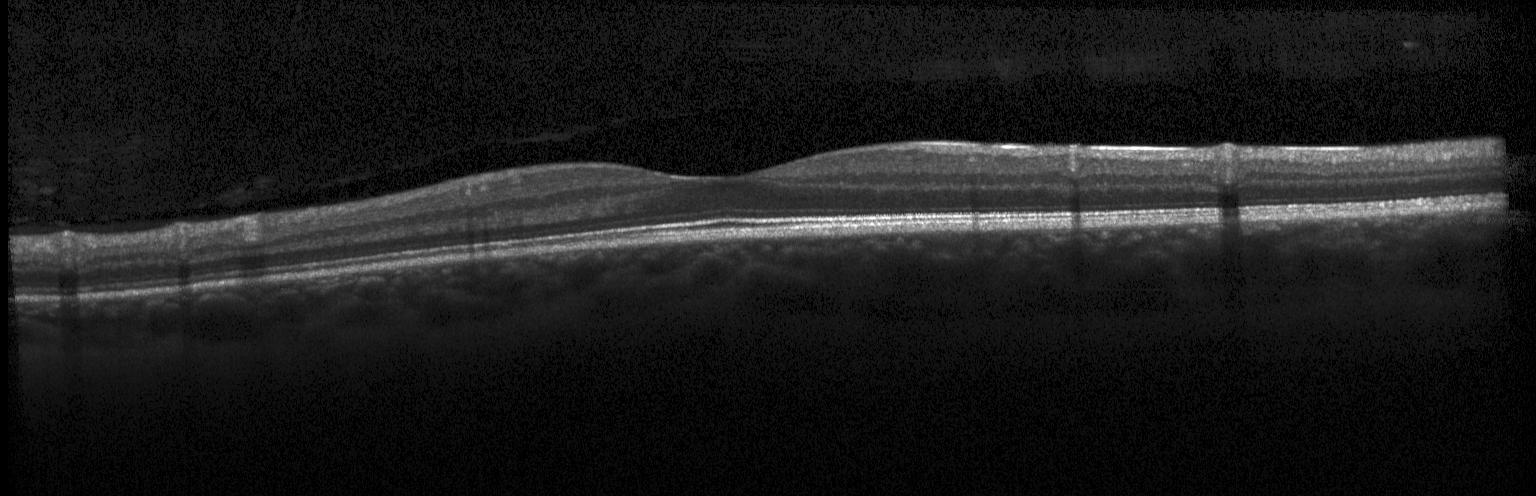 Macular scan. OCT B-scan. Instrument: Heidelberg Spectralis
The scan shows no CNV, DME, or drusen.